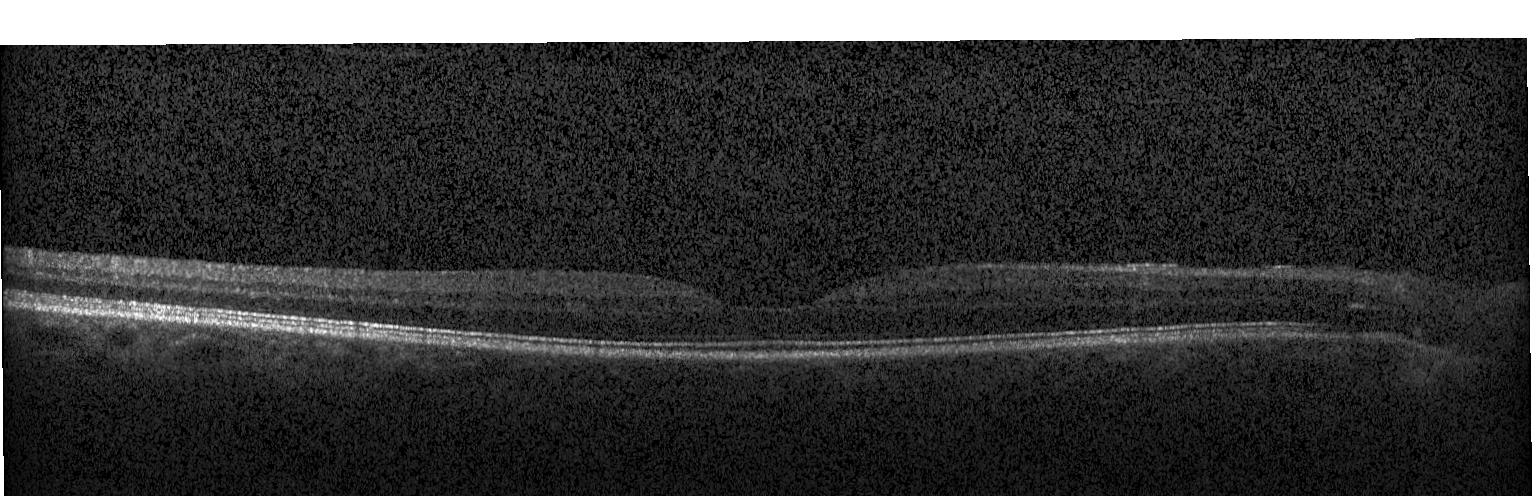 Spectral-domain optical coherence tomography, Heidelberg Spectralis OCT system, fovea-centered, OCT line scan — This B-scan demonstrates no choroidal neovascularization, no diabetic macular edema, and no drusen.